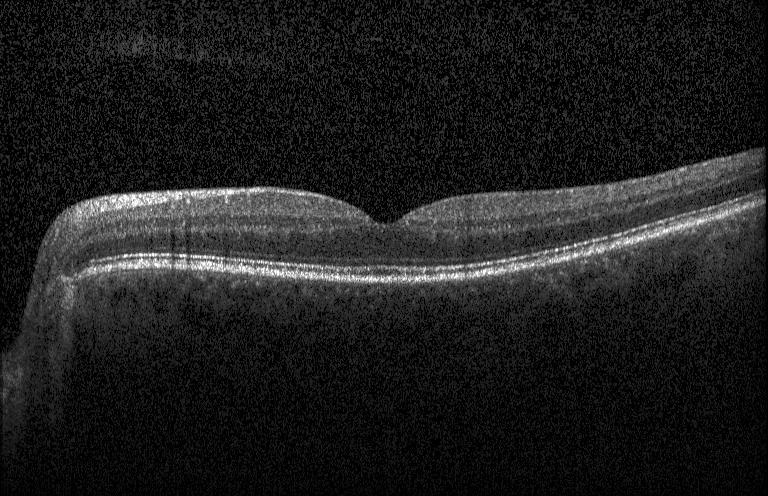 The scan shows no evidence of choroidal neovascularization, diabetic macular edema, or drusen.